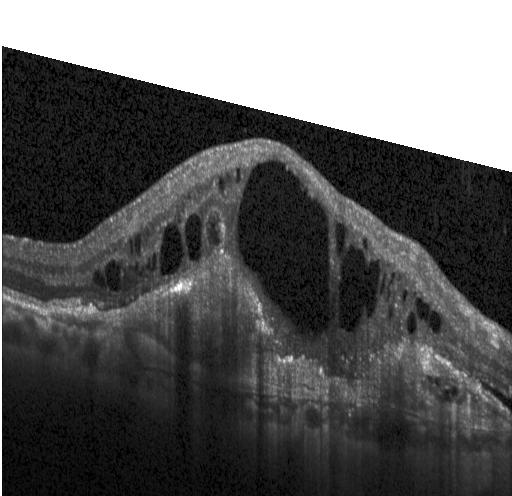 SD-OCT · instrument: Heidelberg Spectralis · retinal OCT B-scan · macular scan — Macular OCT: choroidal neovascularization.